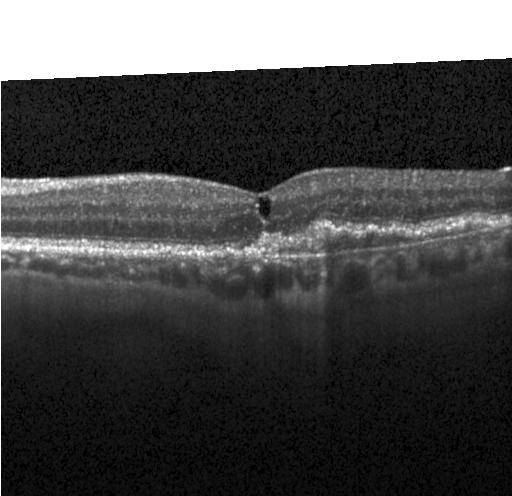
Optical coherence tomography scan — Finding: choroidal neovascularization.